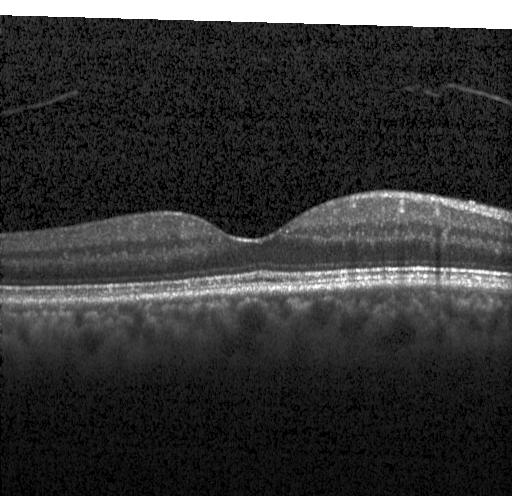
OCT finding: no CNV, no DME, and no drusen.